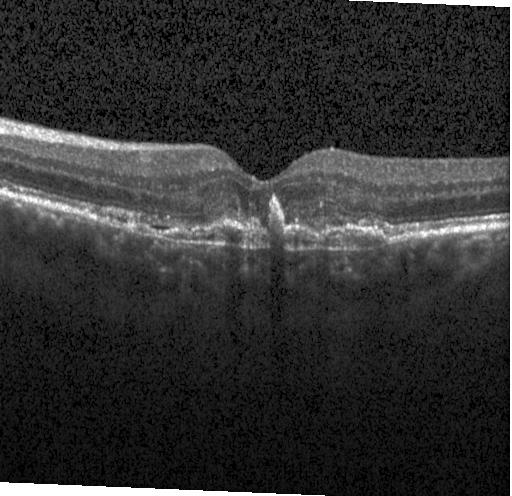 Heidelberg Spectralis · horizontal scan through the fovea · retinal OCT cross-section. This B-scan demonstrates a choroidal neovascular membrane.